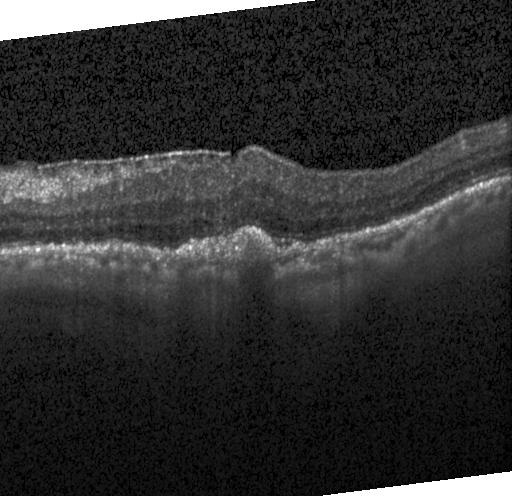

OCT line scan.
The scan shows a choroidal neovascular membrane.